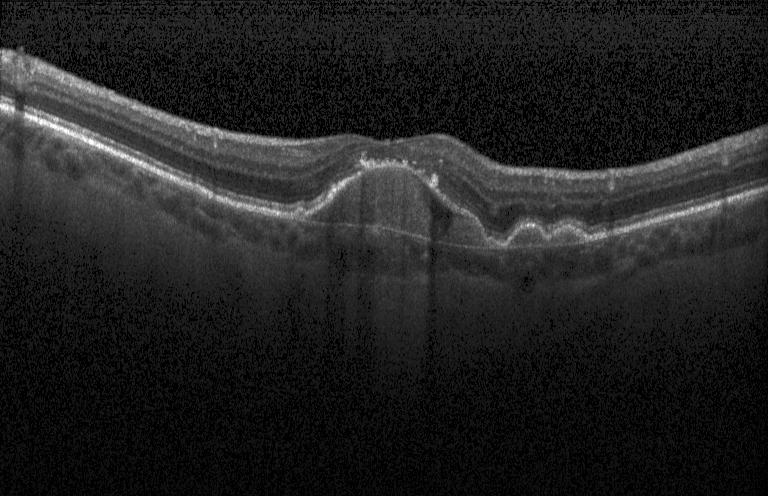
Horizontal scan through the fovea · spectral-domain optical coherence tomography · Heidelberg Spectralis OCT system · optical coherence tomography B-scan. OCT finding: a choroidal neovascular membrane.